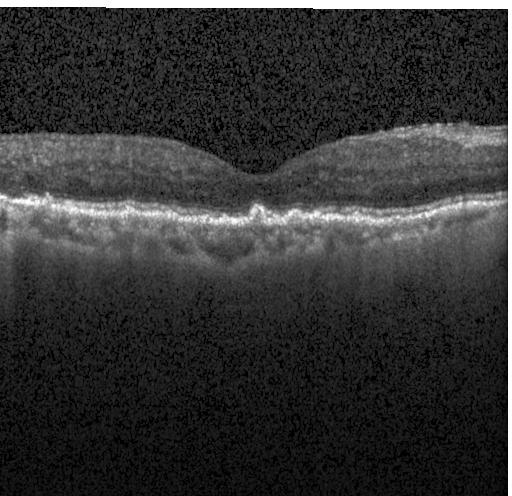

Spectral-domain OCT, acquired on a Heidelberg Spectralis, optical coherence tomography scan. Impression: multiple drusen.